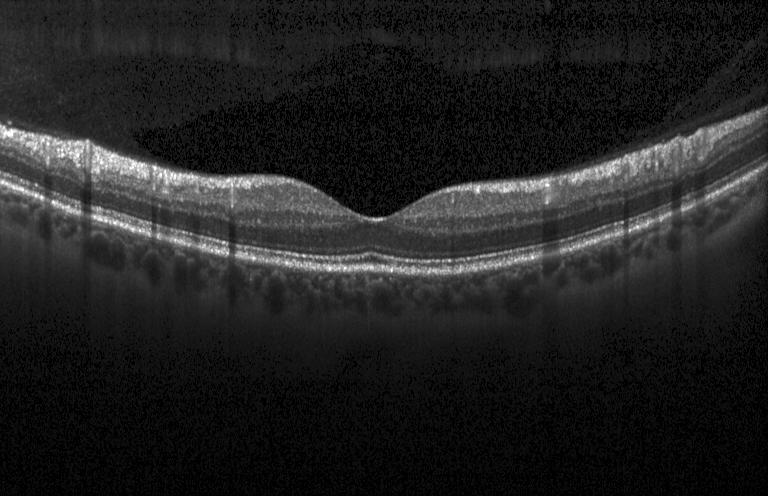 Retinal OCT B-scan · SD-OCT — No CNV, DME, or drusen.